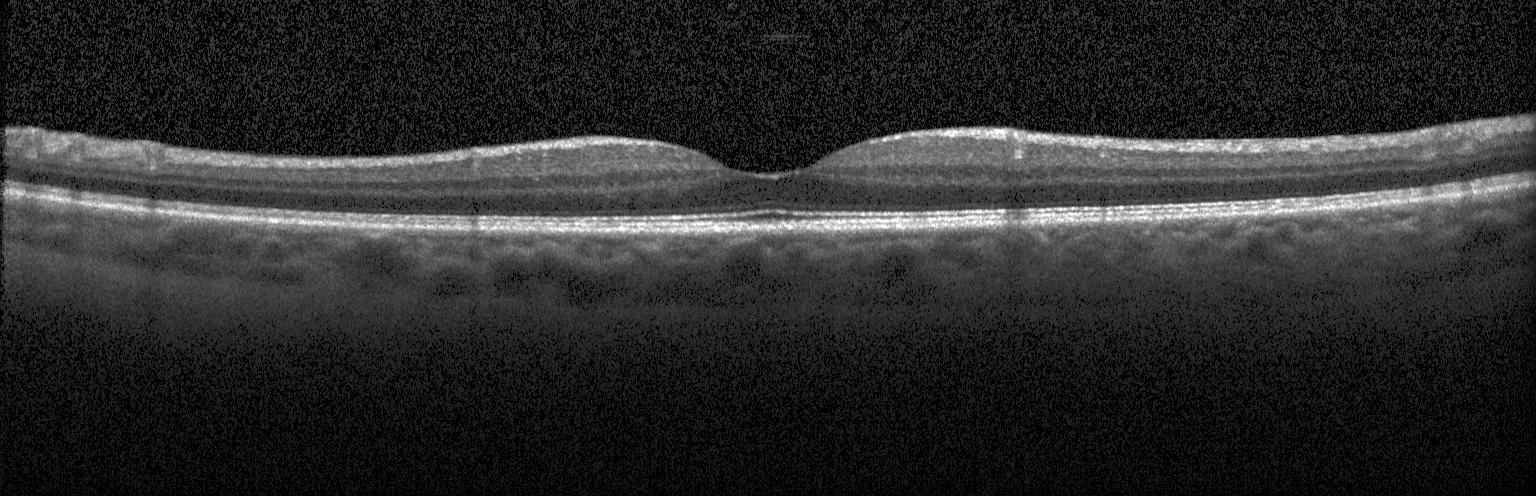

SD-OCT; fovea-centered; instrument: Heidelberg Spectralis; retinal OCT cross-section. Diagnosis: no evidence of choroidal neovascularization, diabetic macular edema, or drusen.